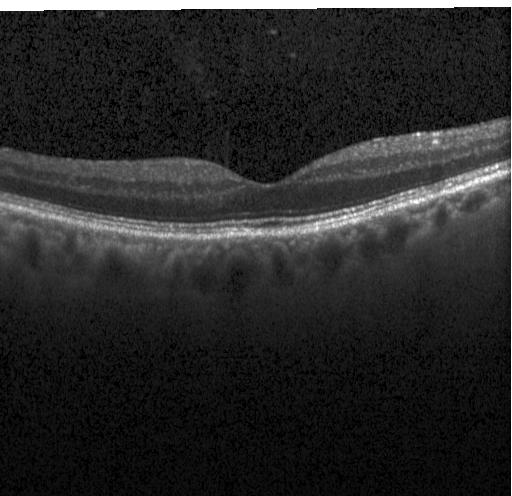 No choroidal neovascularization, no diabetic macular edema, and no drusen.